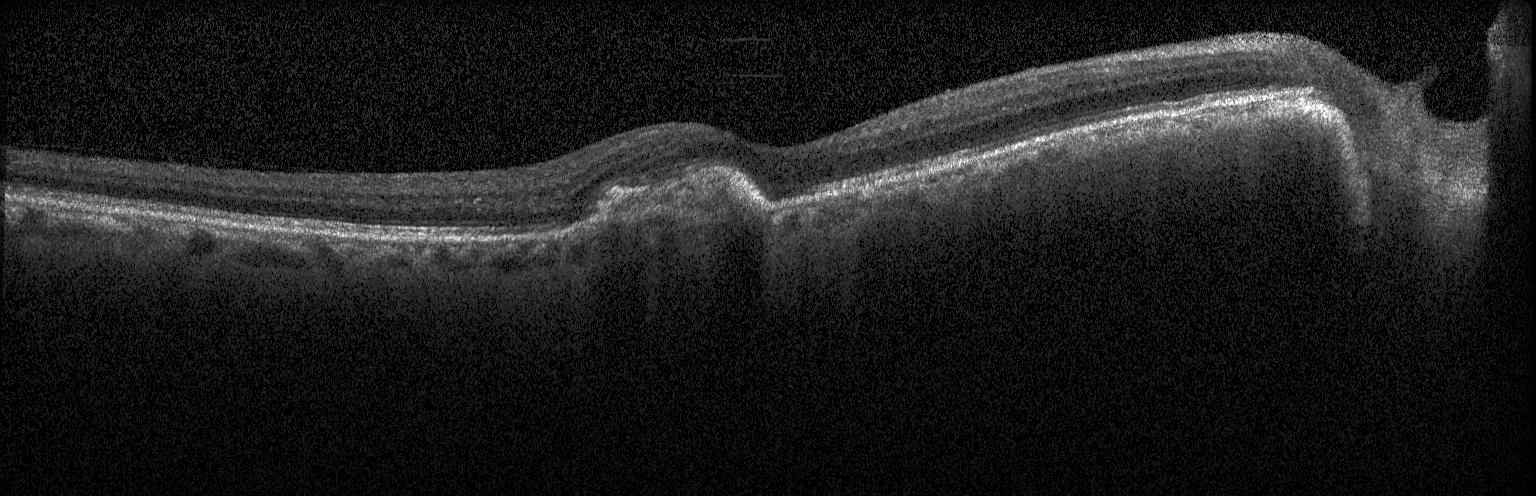 Dx: a choroidal neovascular membrane.